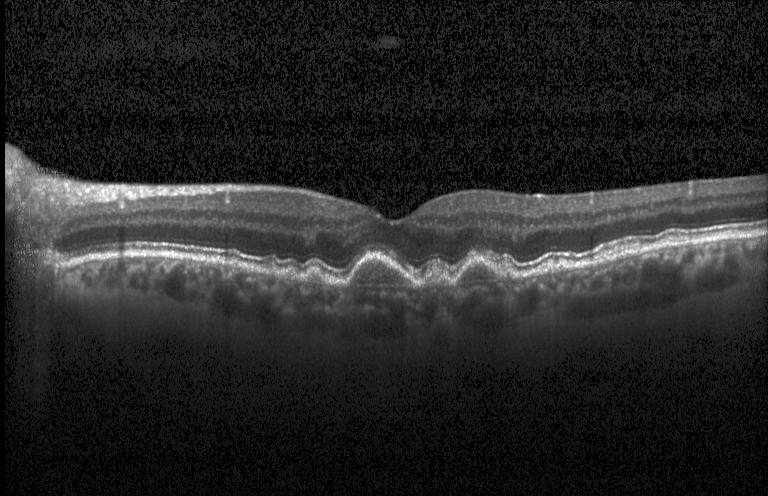
Diagnosis: drusen.